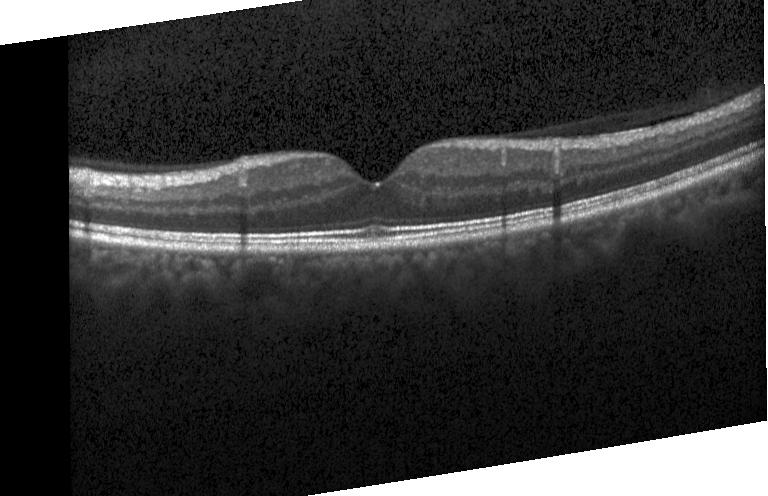

Optical coherence tomography scan. Finding: no CNV, no DME, and no drusen.